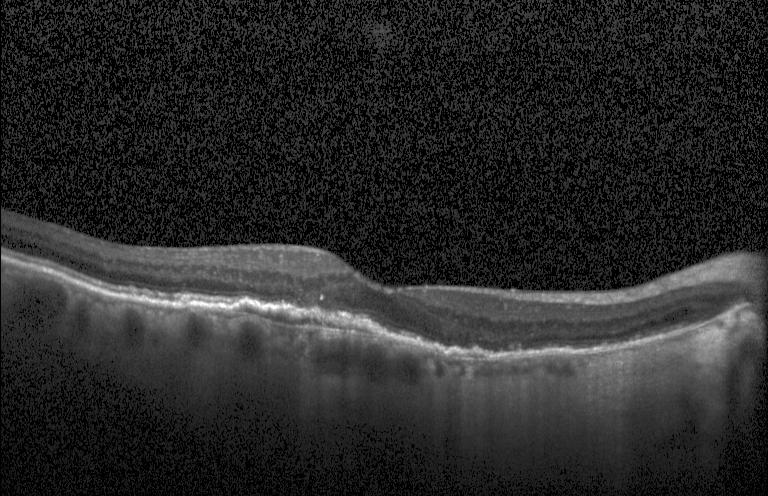
Diagnosis: choroidal neovascularization (CNV).